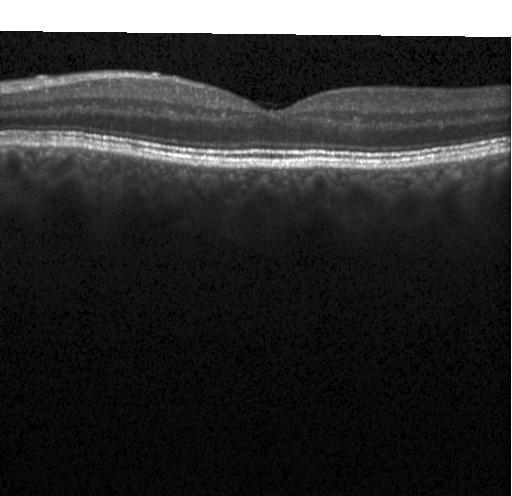
Retinal OCT cross-section. Instrument: Heidelberg Spectralis. SD-OCT — Finding: neither choroidal neovascularization, diabetic macular edema, nor drusen.